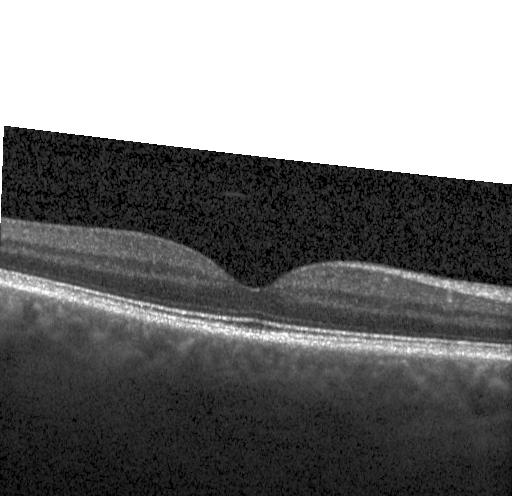 Assessment: neither CNV, DME, nor drusen.